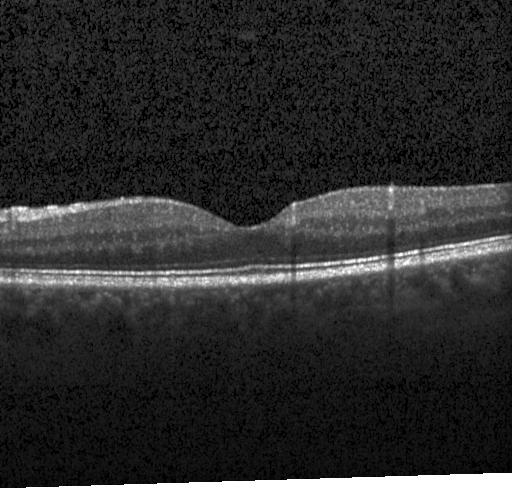

Retinal OCT cross-section showing no choroidal neovascularization, diabetic macular edema, or drusen.